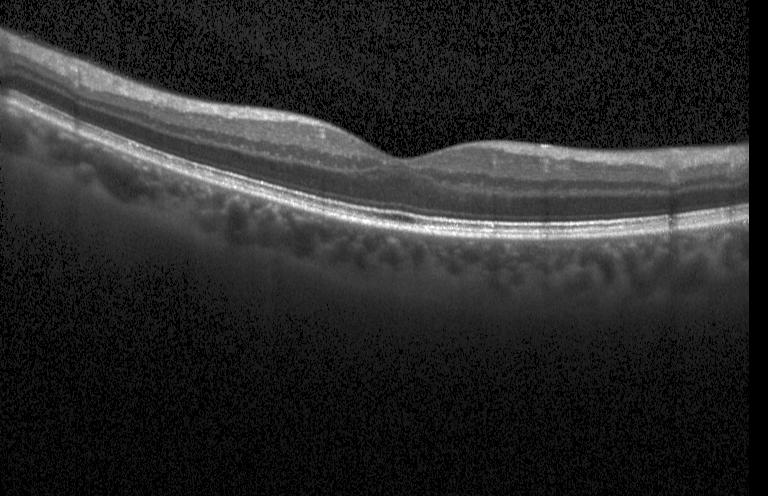

Macular OCT: no evidence of choroidal neovascularization, diabetic macular edema, or drusen.